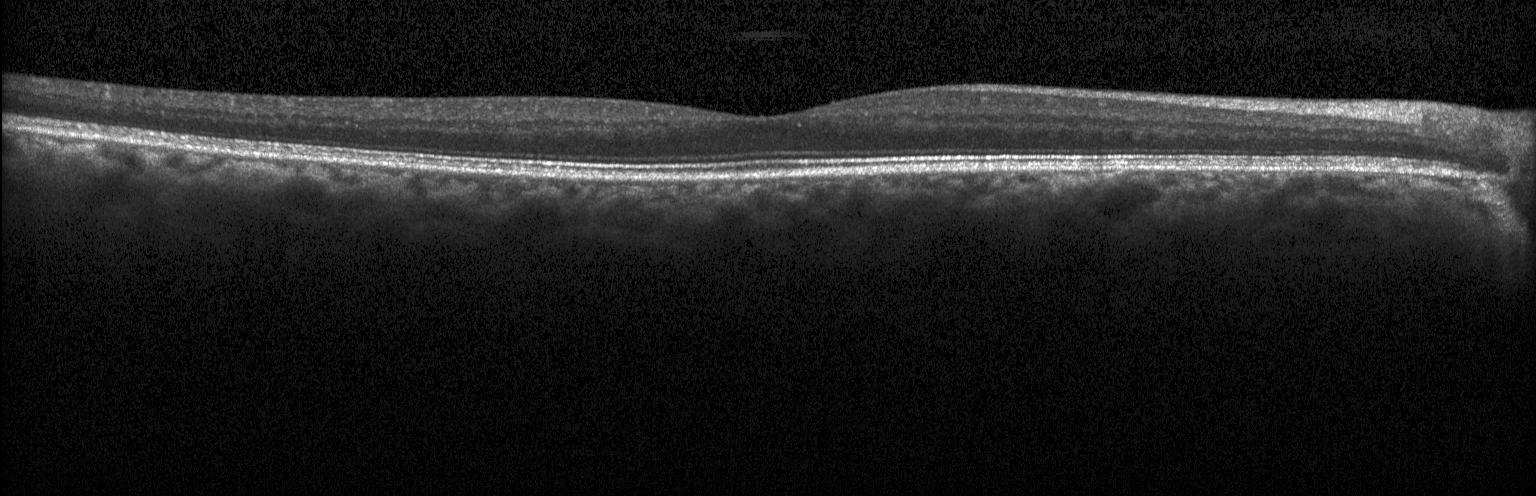
Optical coherence tomography scan; SD-OCT. Impression: neither choroidal neovascularization, diabetic macular edema, nor drusen.